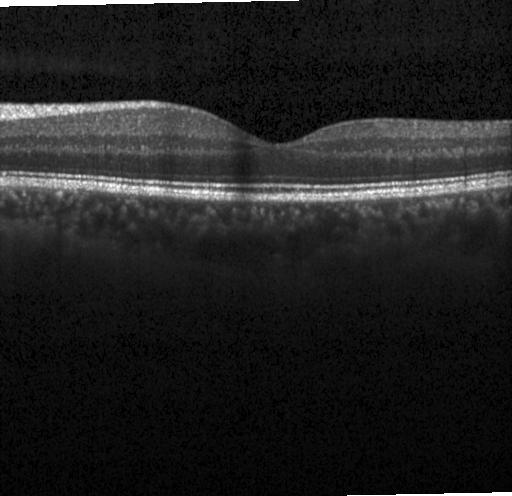 Heidelberg Spectralis · spectral-domain optical coherence tomography · optical coherence tomography scan · horizontal scan through the fovea — Assessment: no CNV, DME, or drusen.